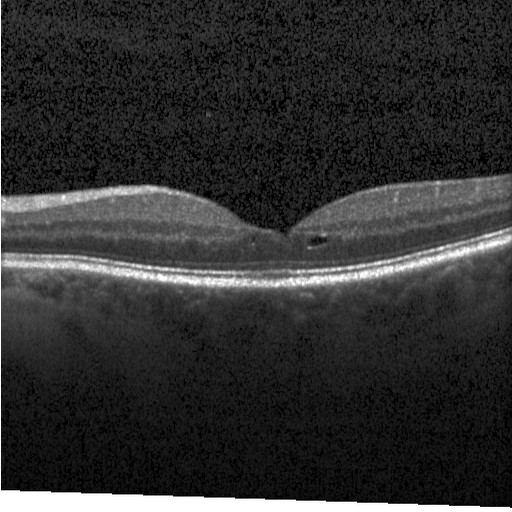
Spectral-domain OCT B-scan: diabetic macular edema (DME).